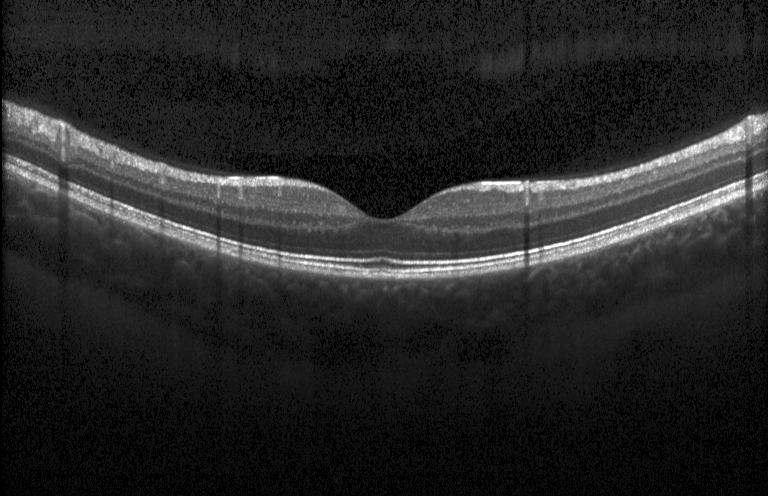
Diagnosis: no evidence of CNV, DME, or drusen.